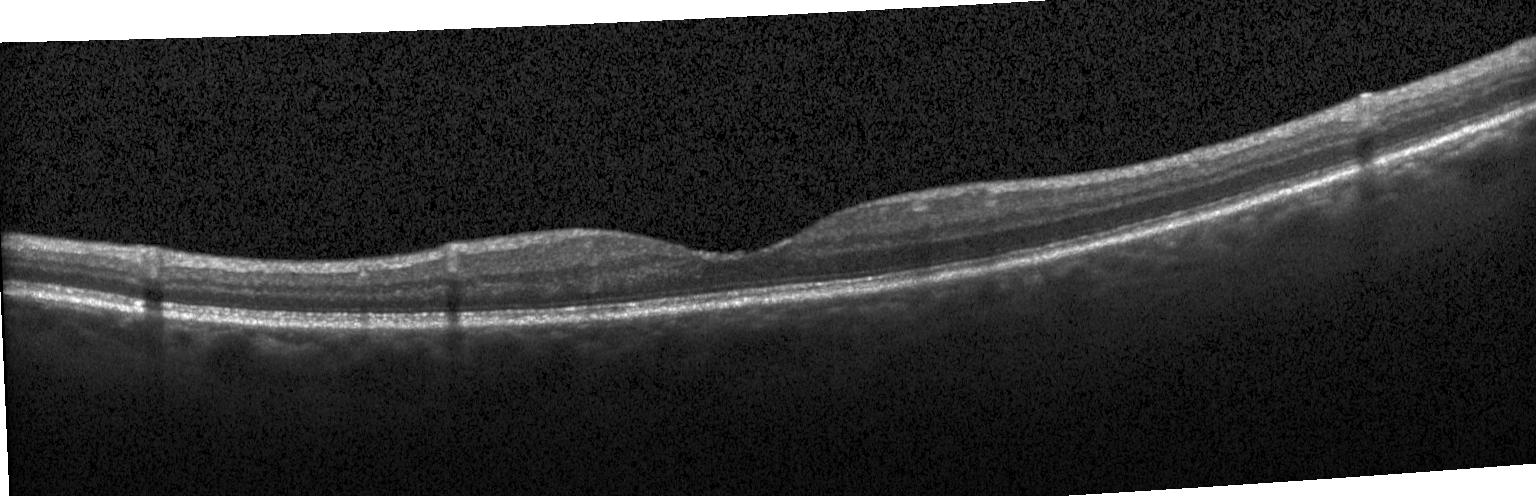

Optical coherence tomography scan. No choroidal neovascularization, no diabetic macular edema, and no drusen.